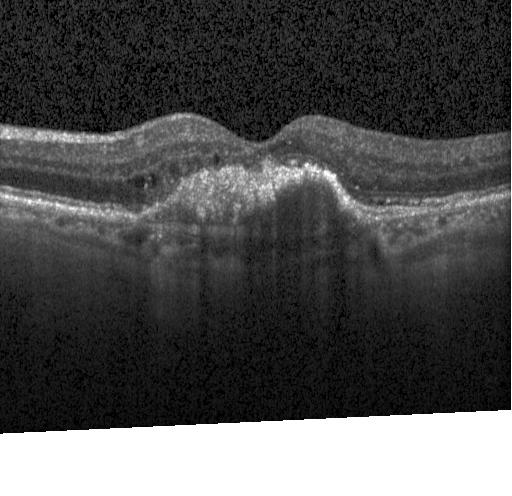
This B-scan demonstrates CNV.